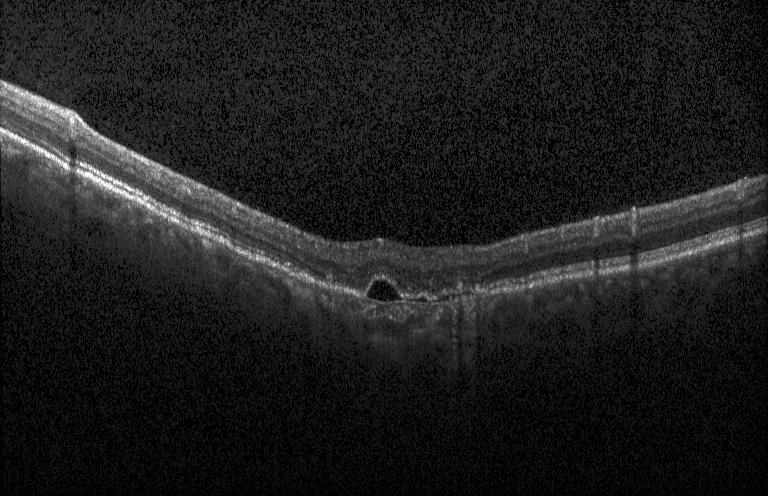
Retinal OCT B-scan. Instrument: Heidelberg Spectralis. Spectral-domain optical coherence tomography. Fovea-centered — This B-scan demonstrates a choroidal neovascular membrane.